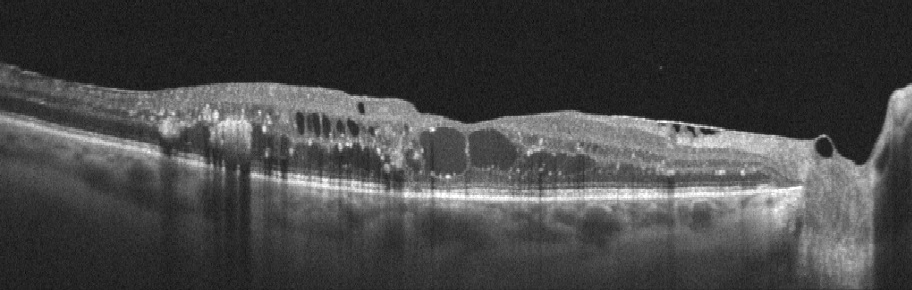 Fovea-centered, instrument: Optovue Avanti RTVue XR, retinal OCT cross-section
OCT finding: DME.